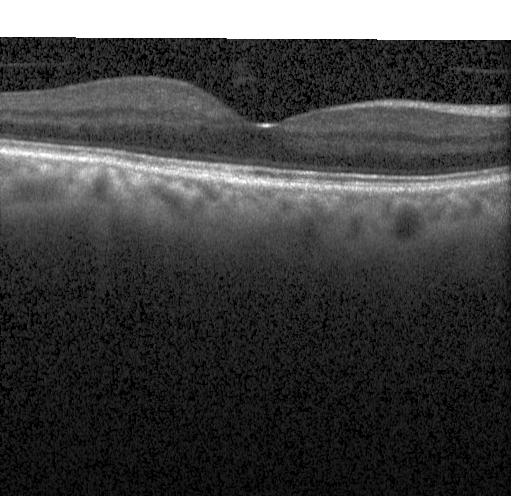 This B-scan demonstrates no CNV, DME, or drusen.